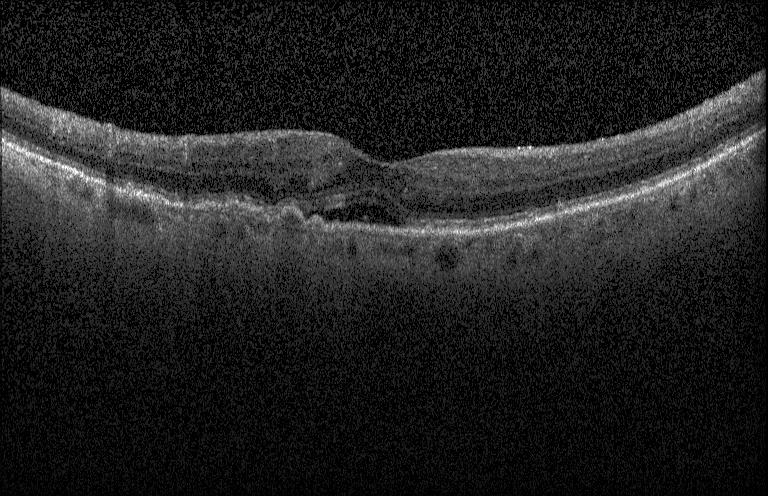 OCT B-scan.
Assessment: CNV.